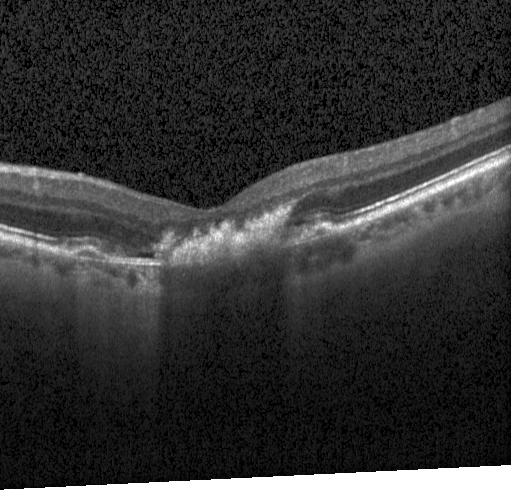

Spectral-domain OCT B-scan: a choroidal neovascular membrane.